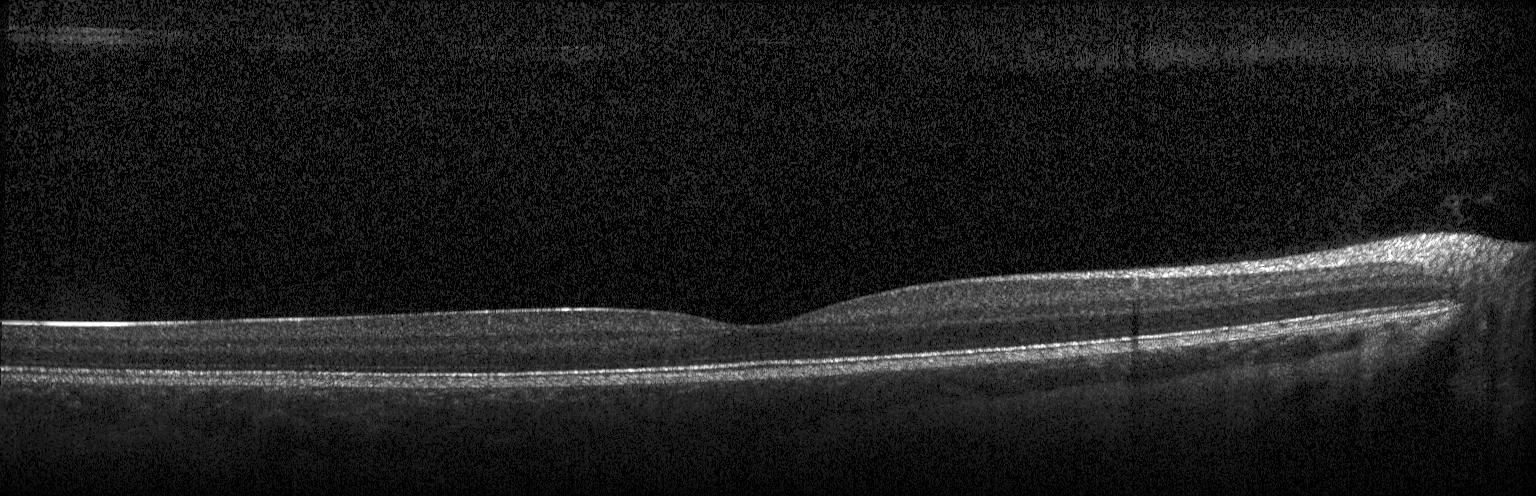
Retinal OCT B-scan — Finding: no choroidal neovascularization, no diabetic macular edema, and no drusen.